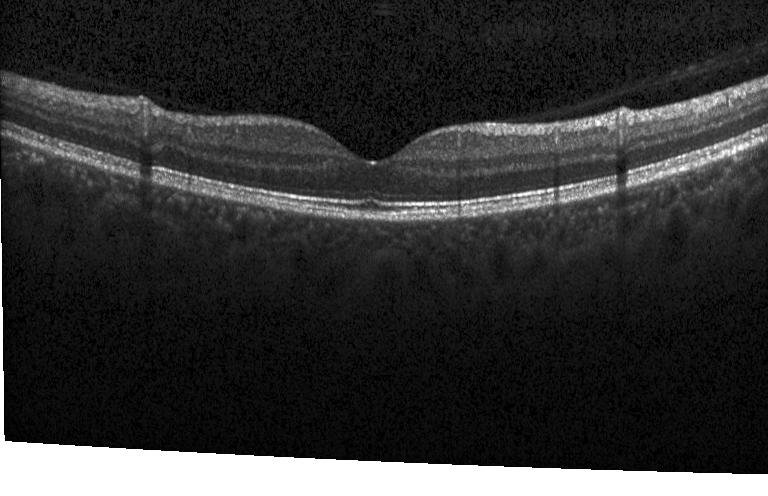
Spectral-domain optical coherence tomography; Heidelberg Spectralis OCT system; retinal OCT B-scan; through the macula. Impression: no choroidal neovascularization, diabetic macular edema, or drusen.